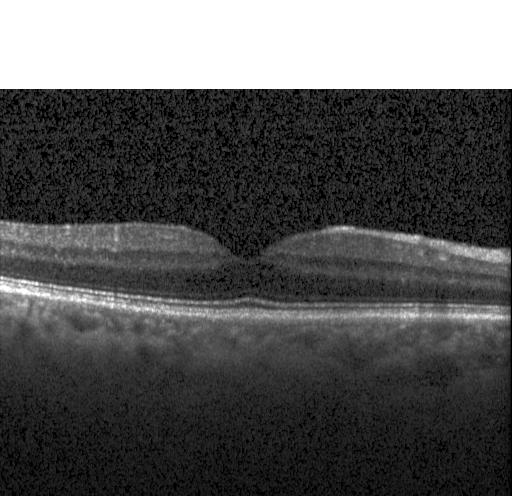 OCT line scan, fovea-centered, SD-OCT
Impression: no choroidal neovascularization, no diabetic macular edema, and no drusen.